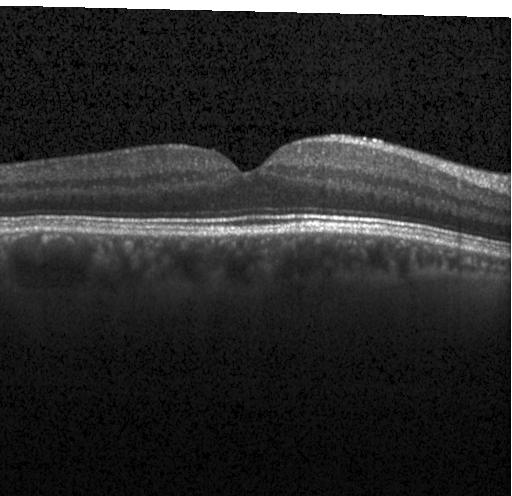
Retinal OCT cross-section · spectral-domain OCT · fovea-centered
Assessment: no CNV, DME, or drusen.